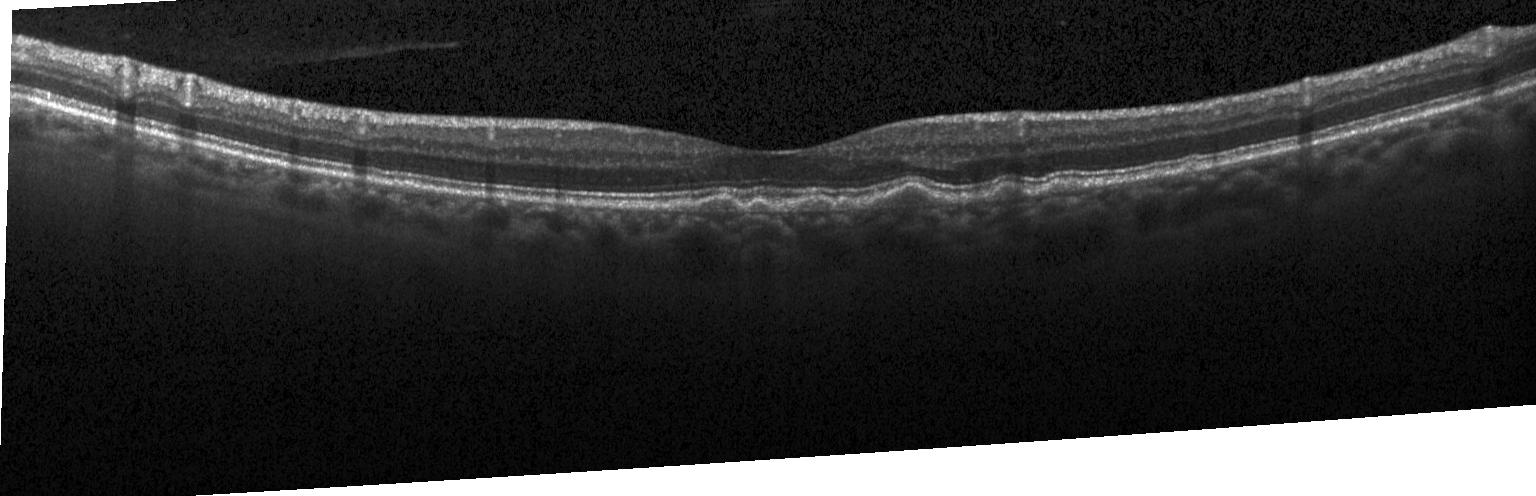

Impression: drusen.